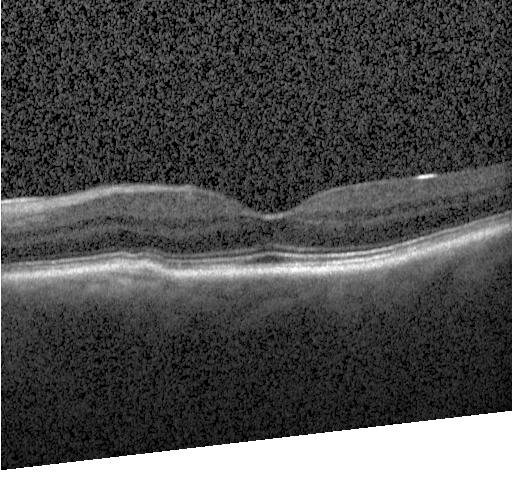

Drusen.